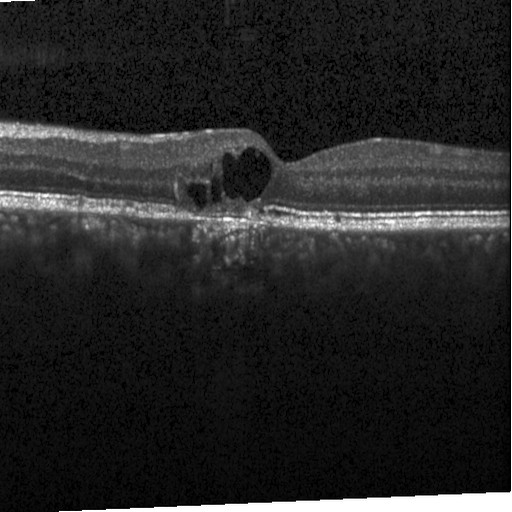

This B-scan demonstrates DME.